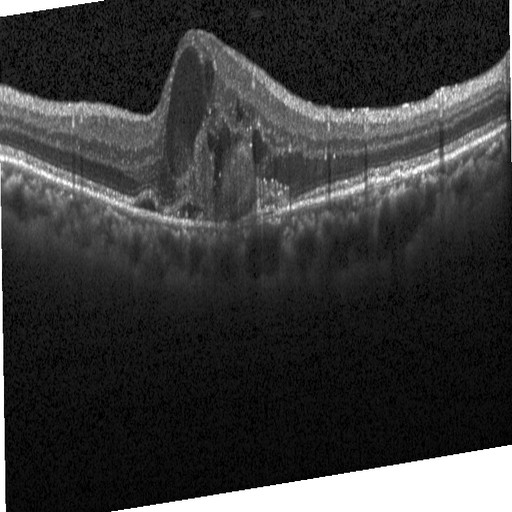

Spectral-domain optical coherence tomography. Retinal OCT cross-section — Impression: diabetic macular edema.